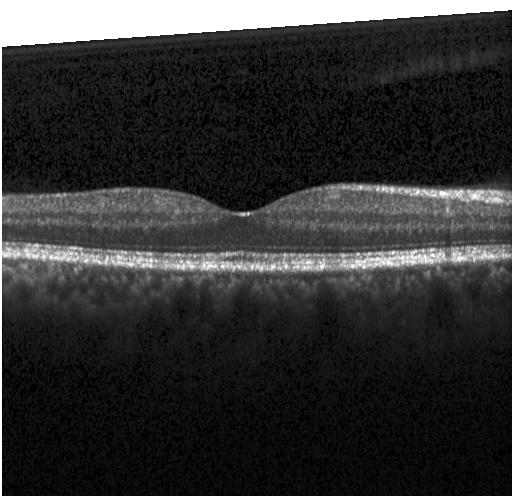 OCT finding: no CNV, no DME, and no drusen.